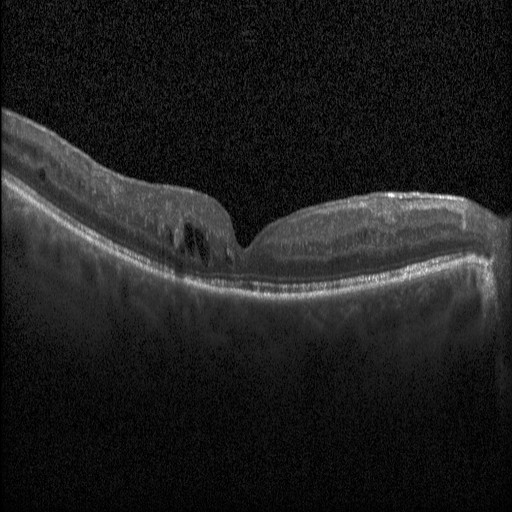
Centered on the fovea. OCT B-scan
Finding: DME.